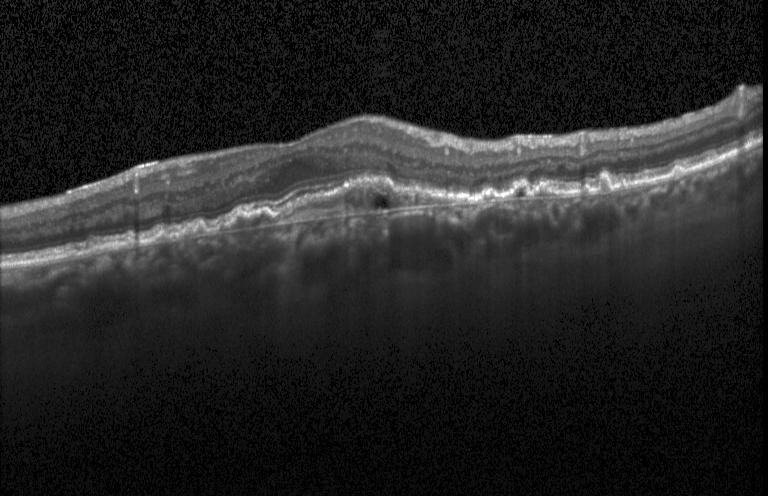

Spectral-domain optical coherence tomography. Centered on the fovea. OCT line scan. Heidelberg Spectralis OCT system — Choroidal neovascularization.